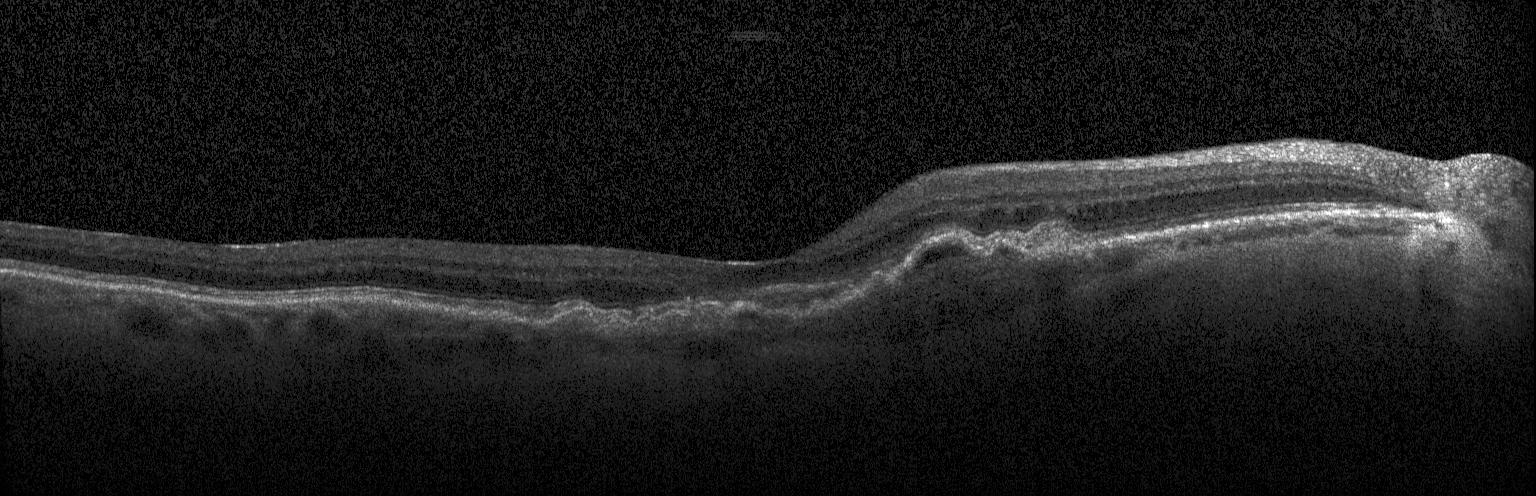
Optical coherence tomography B-scan; fovea-centered. OCT finding: a choroidal neovascular membrane.